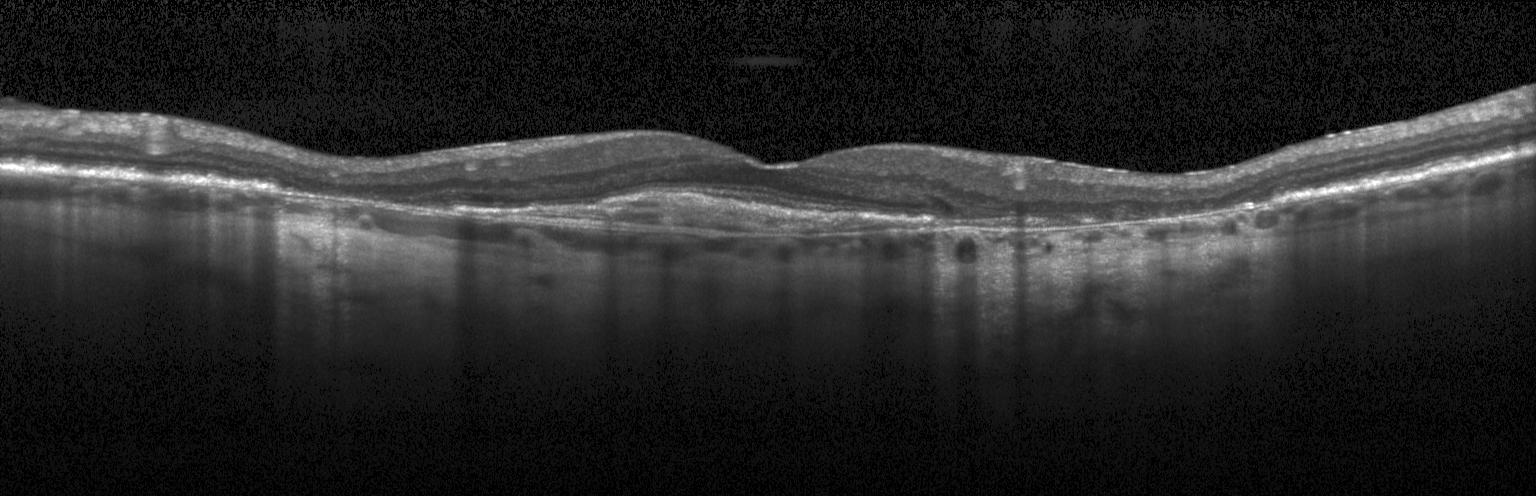 OCT line scan. Macular OCT: choroidal neovascularization.